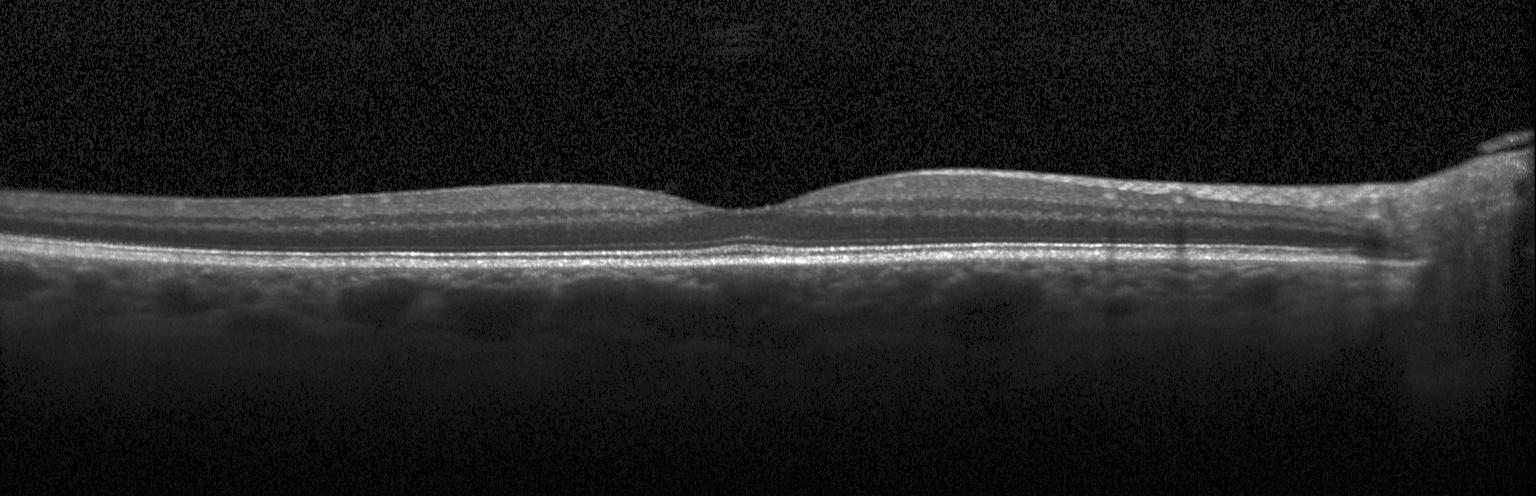

Optical coherence tomography scan, spectral-domain optical coherence tomography, fovea-centered.
Impression: no choroidal neovascularization, diabetic macular edema, or drusen.